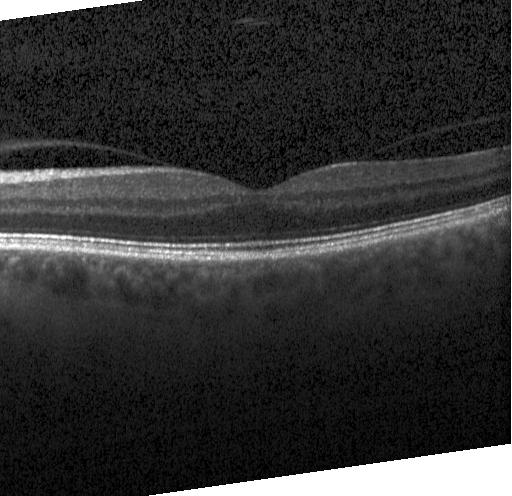

Fovea-centered. Heidelberg Spectralis OCT system. SD-OCT. Retinal OCT cross-section
Impression: no CNV, DME, or drusen.